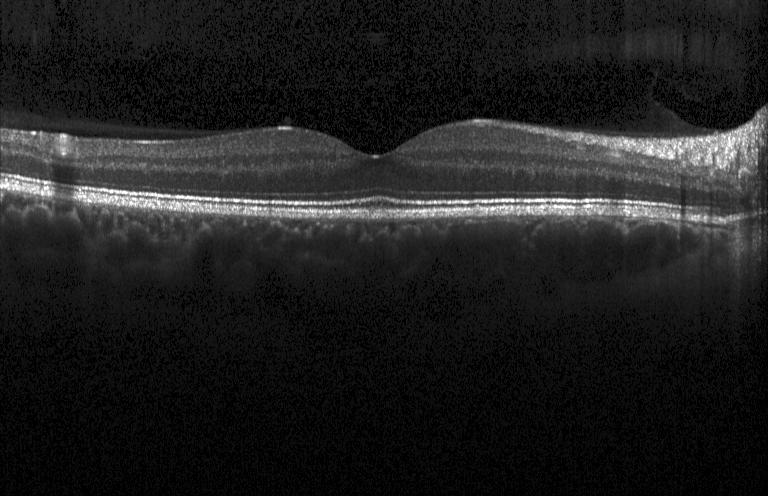

OCT line scan. OCT finding: neither CNV, DME, nor drusen.